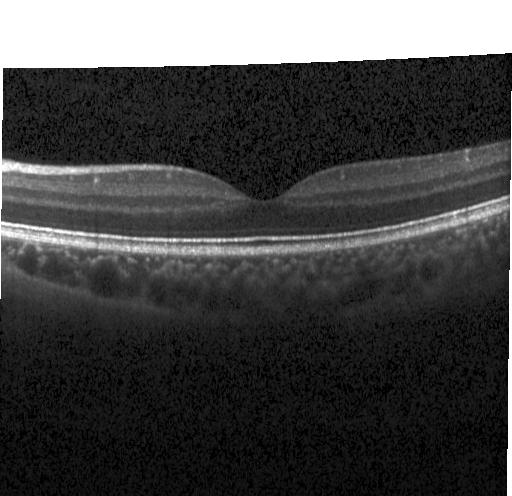
Optical coherence tomography B-scan. Heidelberg Spectralis. Assessment: no CNV, no DME, and no drusen.